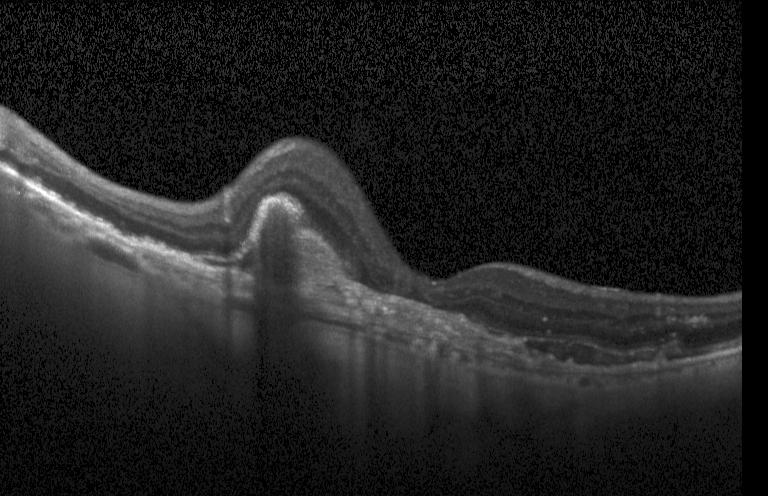

OCT B-scan. Instrument: Heidelberg Spectralis. Spectral-domain OCT.
Diagnosis: a choroidal neovascular membrane.